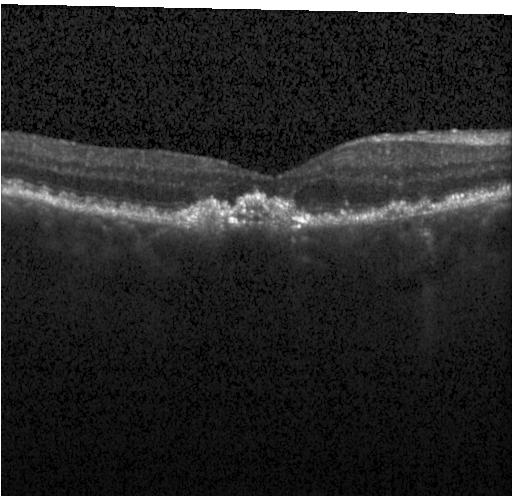
The scan shows a choroidal neovascular membrane.